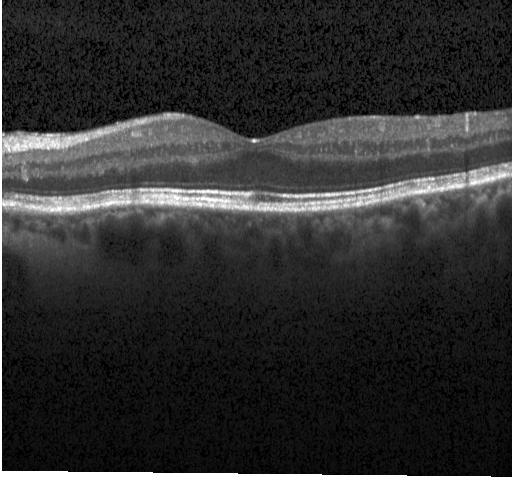

Finding: no choroidal neovascularization, no diabetic macular edema, and no drusen.